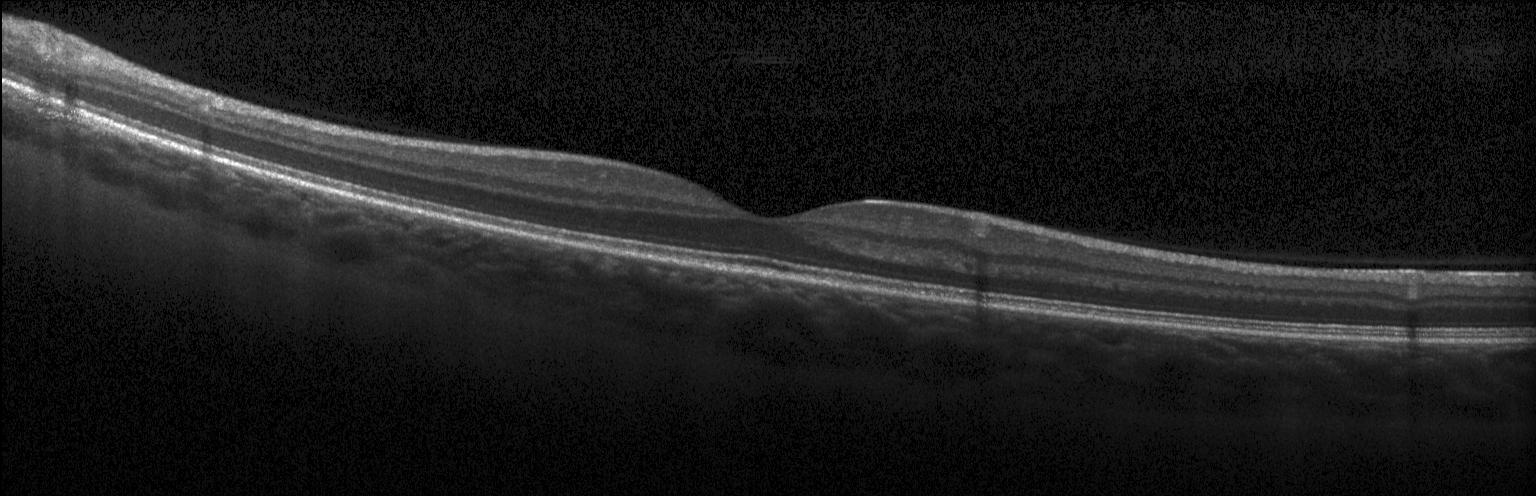
Retinal OCT cross-section. Through the macula.
Dx: neither CNV, DME, nor drusen.